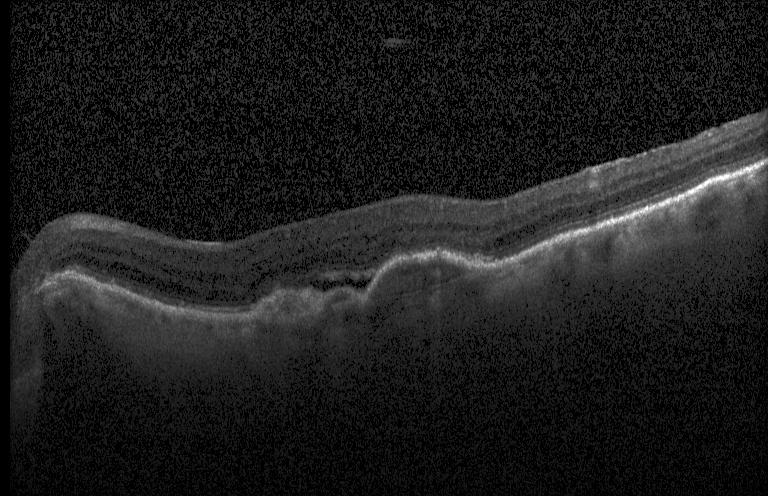 Spectral-domain OCT. Optical coherence tomography B-scan.
Impression: a choroidal neovascular membrane.